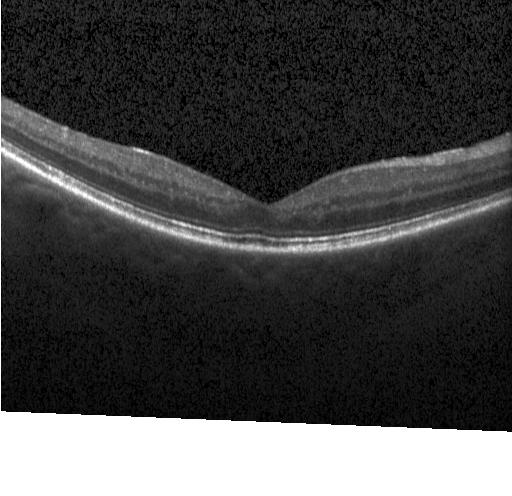
Spectral-domain OCT; retinal OCT cross-section; through the macula; Heidelberg Spectralis OCT system.
Neither choroidal neovascularization, diabetic macular edema, nor drusen.